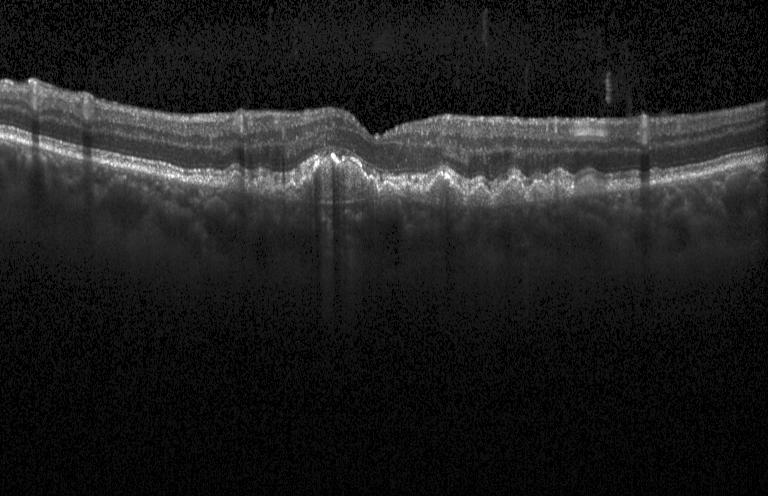

Spectral-domain optical coherence tomography, retinal OCT cross-section.
Diagnosis: a choroidal neovascular membrane.